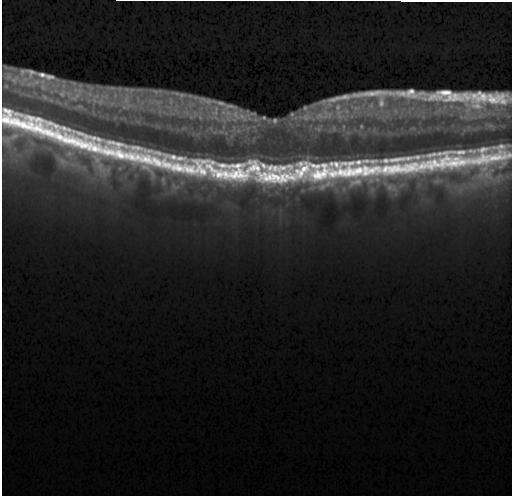
Diagnosis: drusen.